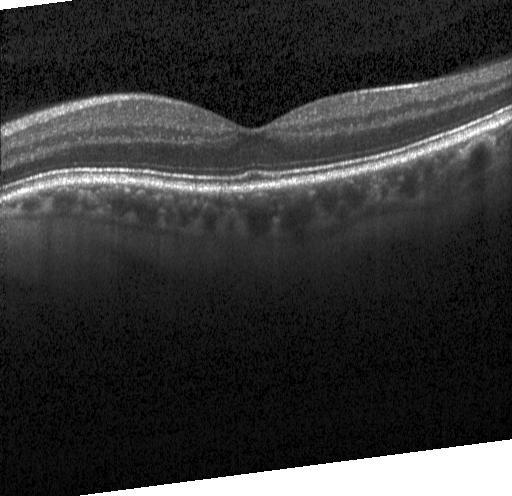

Diagnosis: no CNV, DME, or drusen.